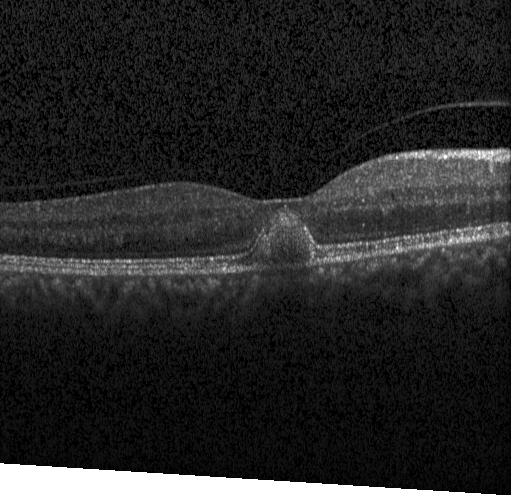 OCT finding: choroidal neovascularization.